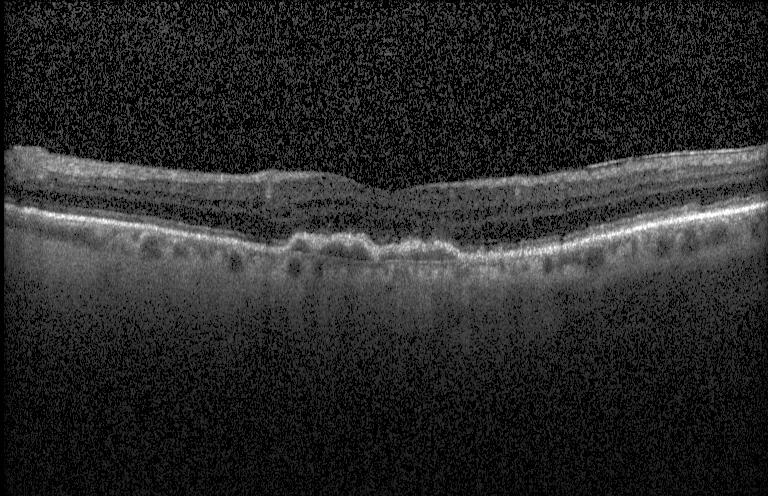 Fovea-centered. Instrument: Heidelberg Spectralis. Retinal OCT B-scan — Finding: a choroidal neovascular membrane.